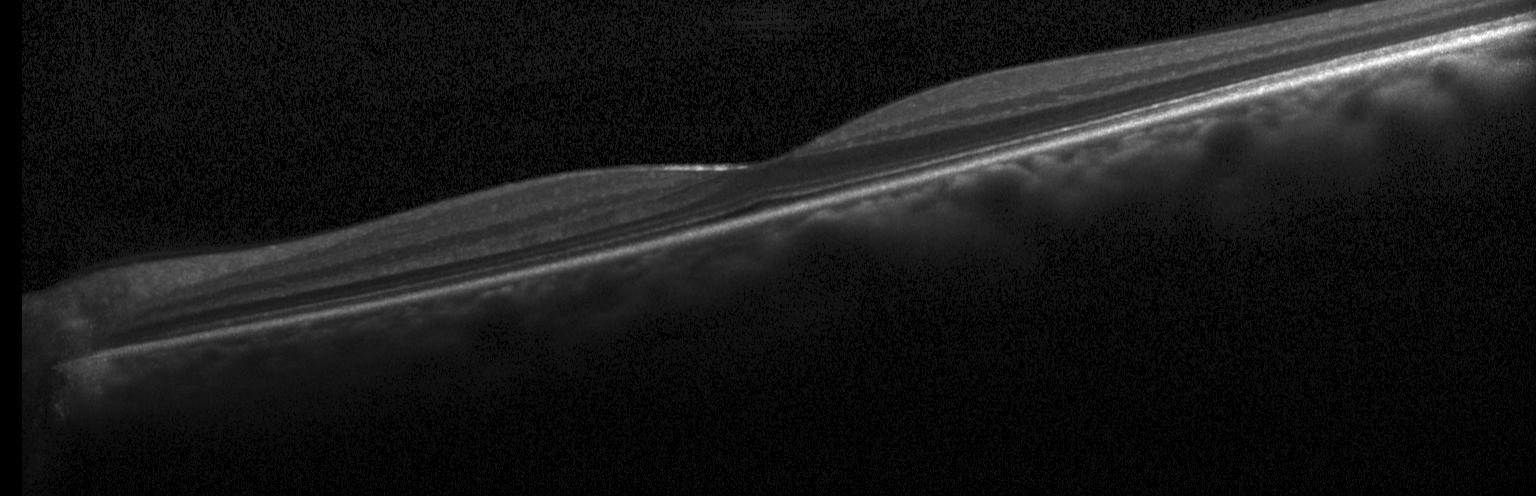
Retinal OCT cross-section · acquired on a Heidelberg Spectralis.
Finding: neither CNV, DME, nor drusen.